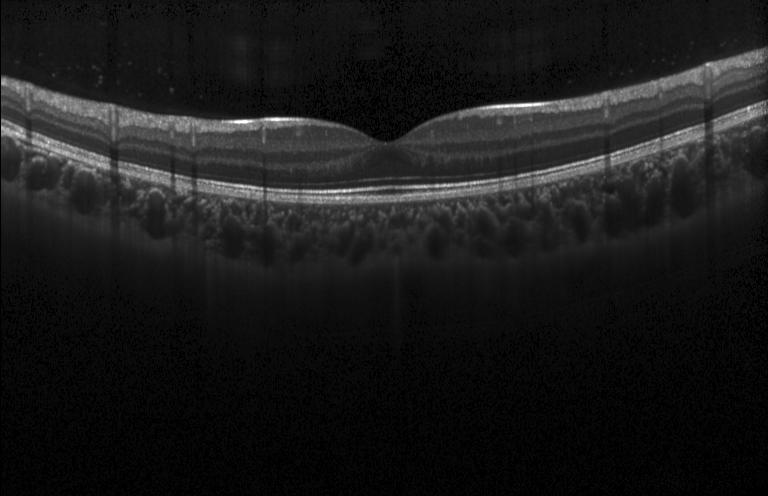 Heidelberg Spectralis OCT system. Optical coherence tomography scan. Fovea-centered — Macular OCT: neither choroidal neovascularization, diabetic macular edema, nor drusen.